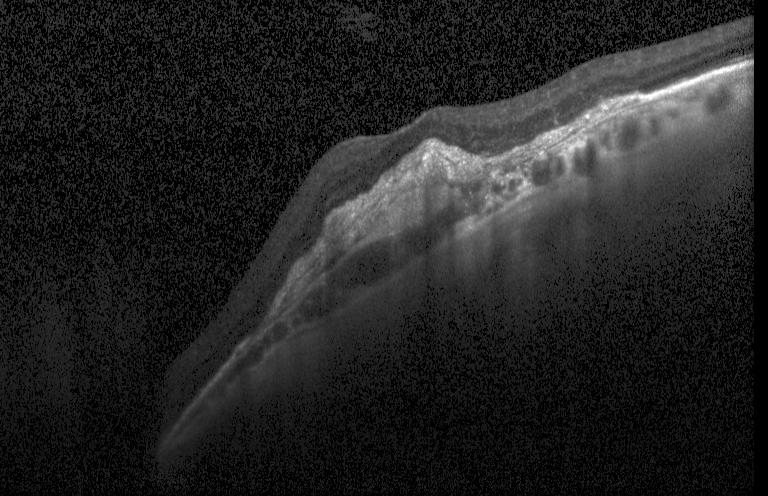
Retinal OCT B-scan; spectral-domain OCT. This B-scan demonstrates a choroidal neovascular membrane.